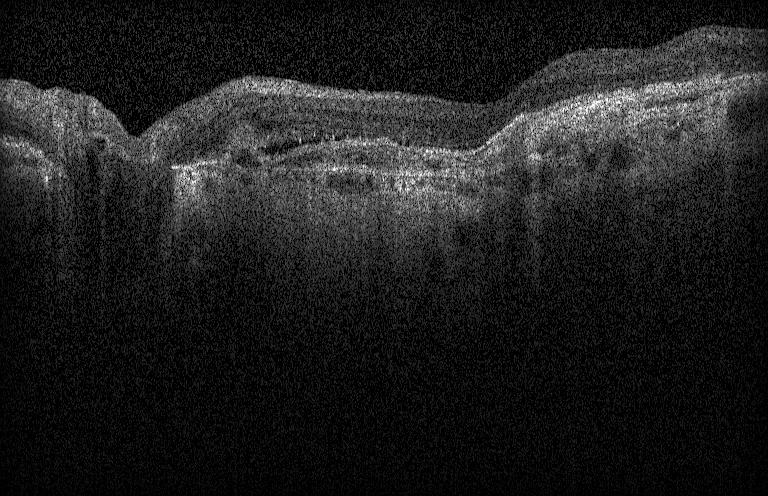
Optical coherence tomography scan
Diagnosis: a choroidal neovascular membrane.